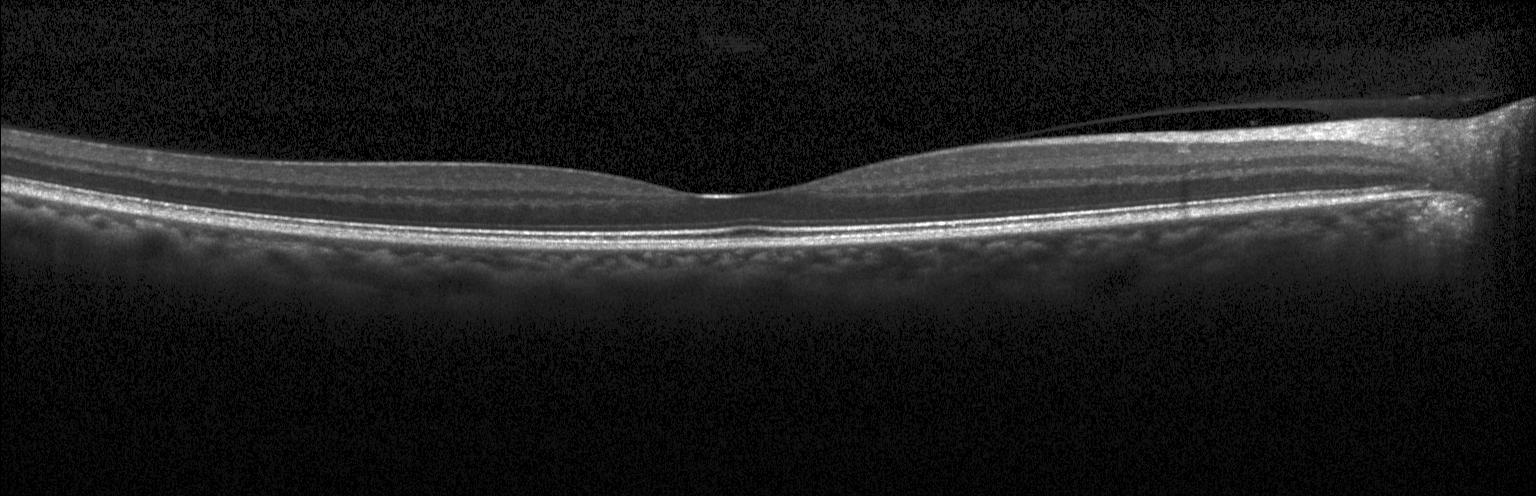
Optical coherence tomography scan. This B-scan demonstrates no choroidal neovascularization, no diabetic macular edema, and no drusen.